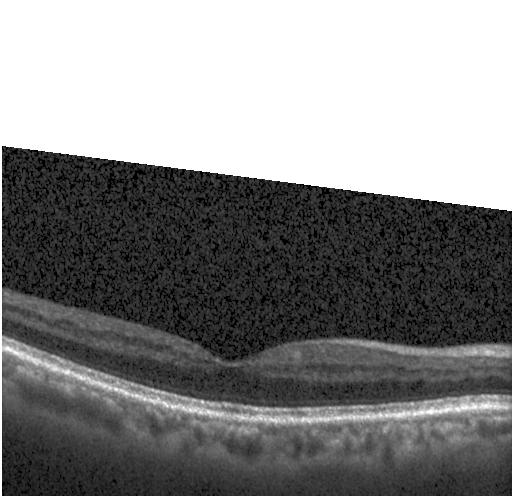
Optical coherence tomography B-scan.
No choroidal neovascularization, diabetic macular edema, or drusen.